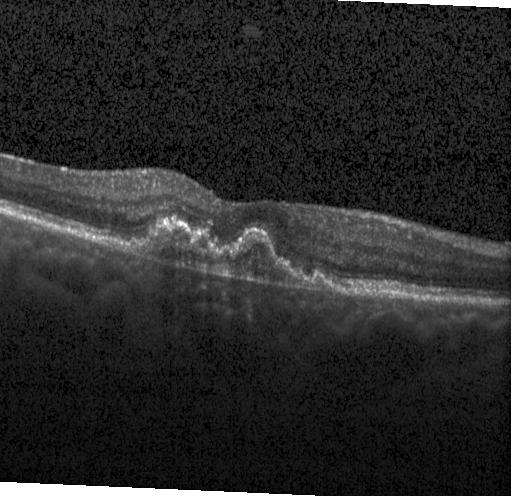 Horizontal scan through the fovea · retinal OCT B-scan · Heidelberg Spectralis · spectral-domain OCT. OCT finding: a choroidal neovascular membrane.